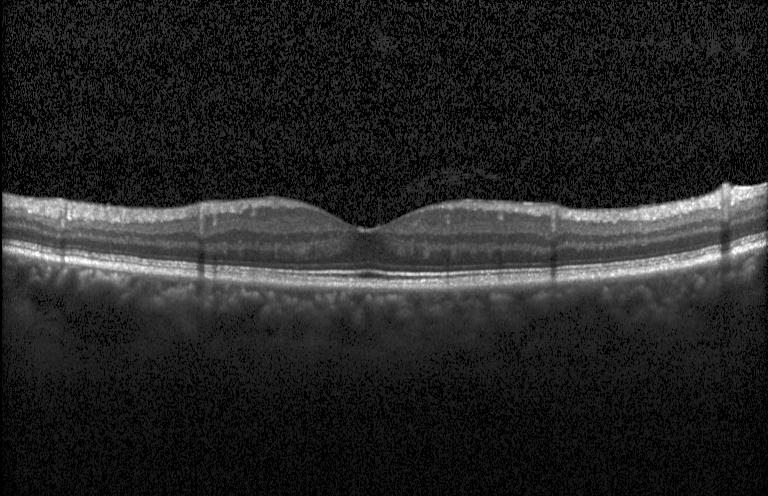 Retinal OCT cross-section. Diagnosis: no evidence of choroidal neovascularization, diabetic macular edema, or drusen.